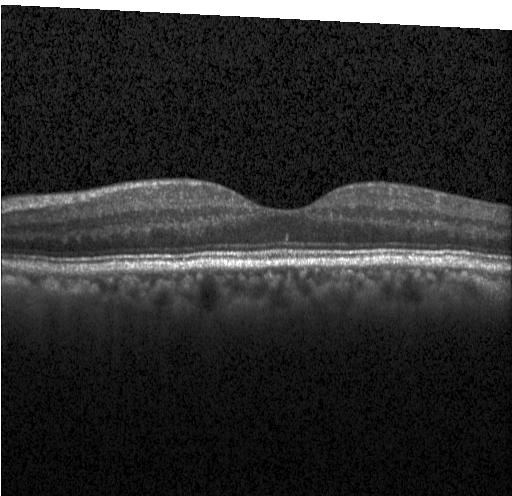 OCT B-scan. SD-OCT. Fovea-centered. Instrument: Heidelberg Spectralis — Macular OCT: no CNV, no DME, and no drusen.